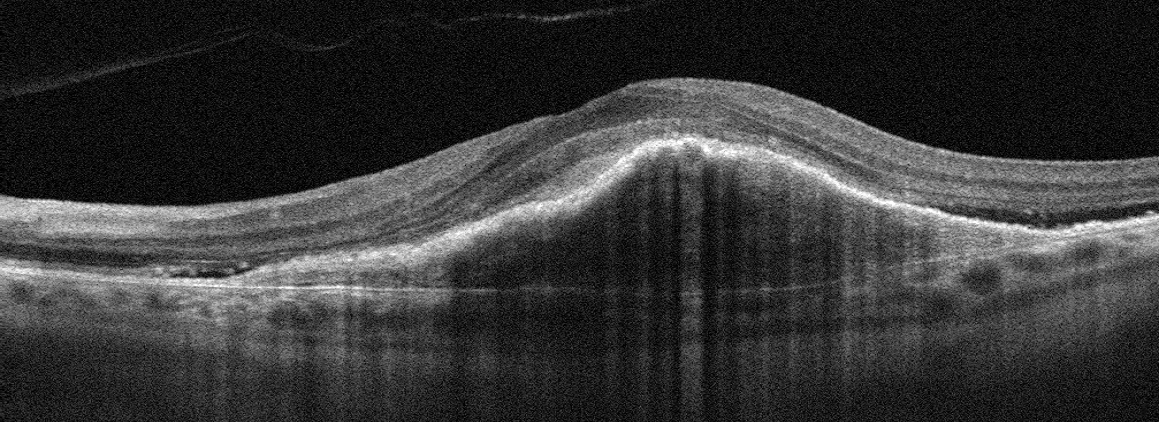
Left eye; OCT B-scan. Impression: AMD.